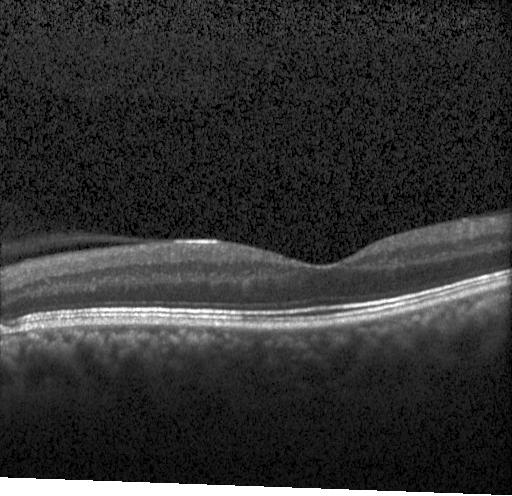 SD-OCT, retinal OCT B-scan, macular scan, Heidelberg Spectralis OCT system. Diagnosis: no choroidal neovascularization, diabetic macular edema, or drusen.